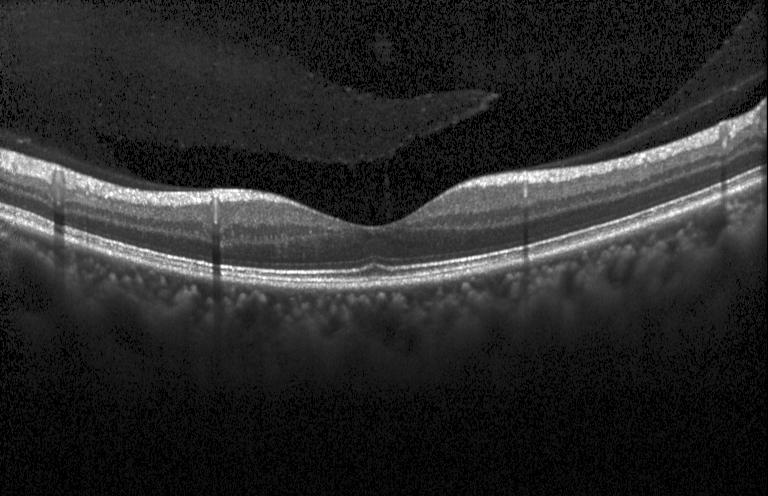
OCT scan showing no choroidal neovascularization, diabetic macular edema, or drusen.